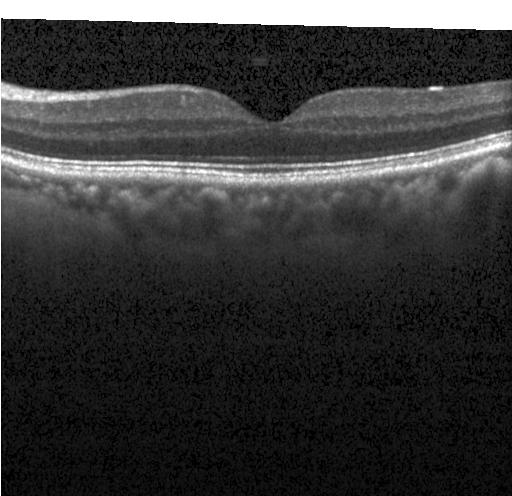
Instrument: Heidelberg Spectralis. Optical coherence tomography scan
Dx: neither choroidal neovascularization, diabetic macular edema, nor drusen.